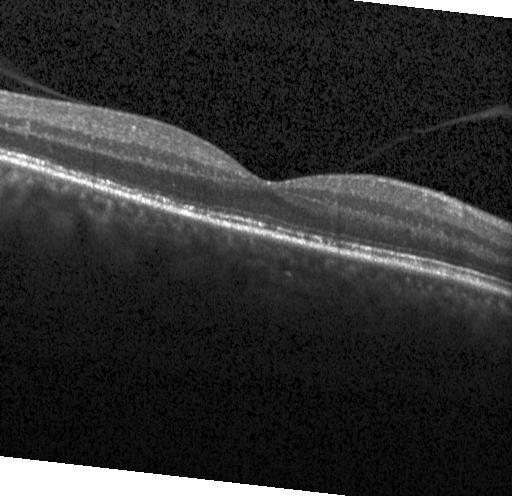 OCT line scan. Impression: no CNV, DME, or drusen.